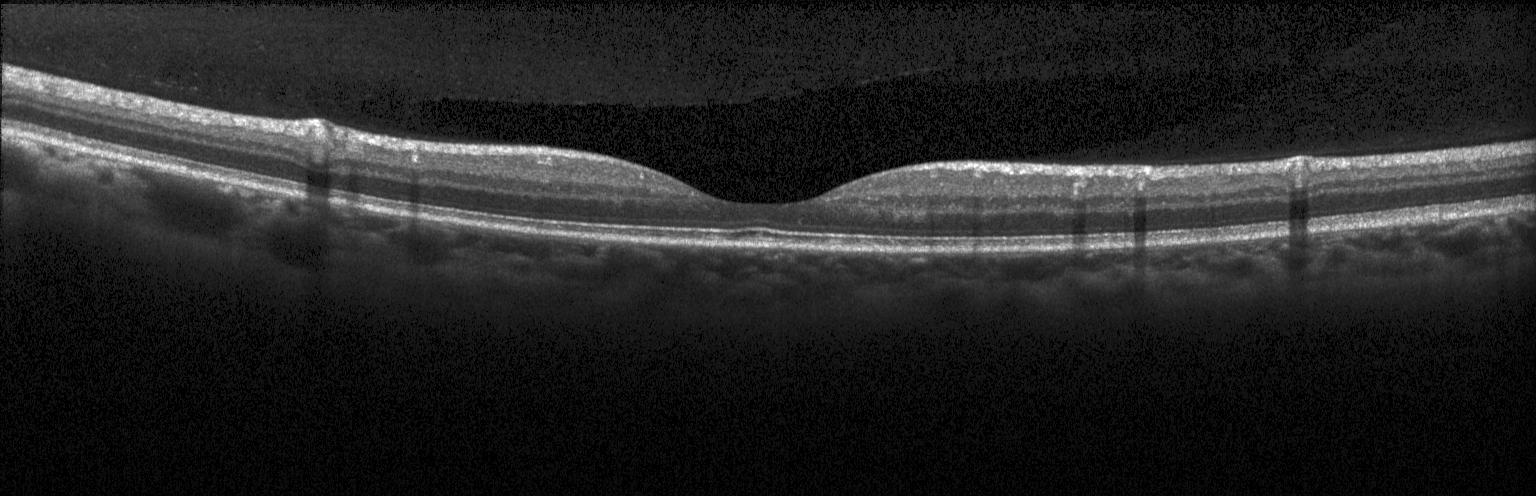
Instrument: Heidelberg Spectralis · horizontal scan through the fovea · retinal OCT cross-section.
Impression: neither choroidal neovascularization, diabetic macular edema, nor drusen.